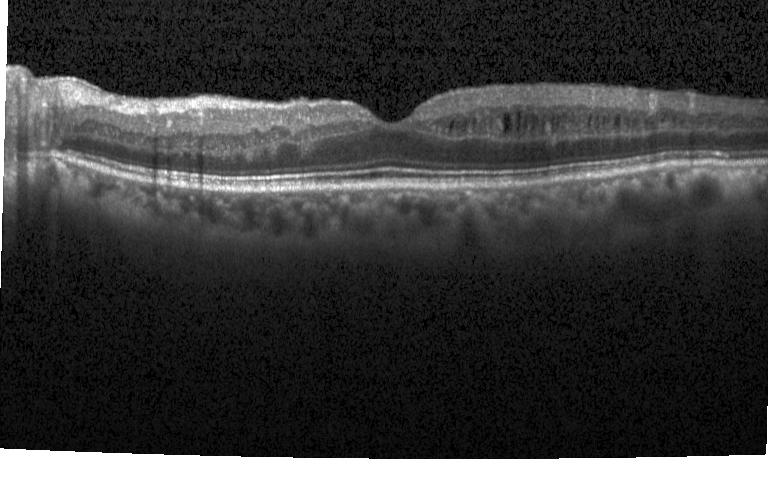 Macular OCT: diabetic macular edema (DME).